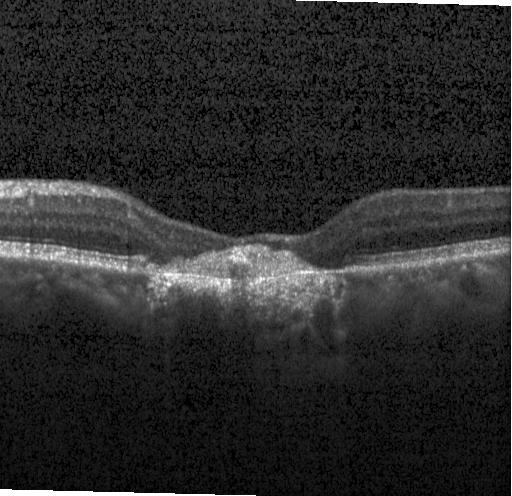 Optical coherence tomography B-scan. This B-scan demonstrates a choroidal neovascular membrane.